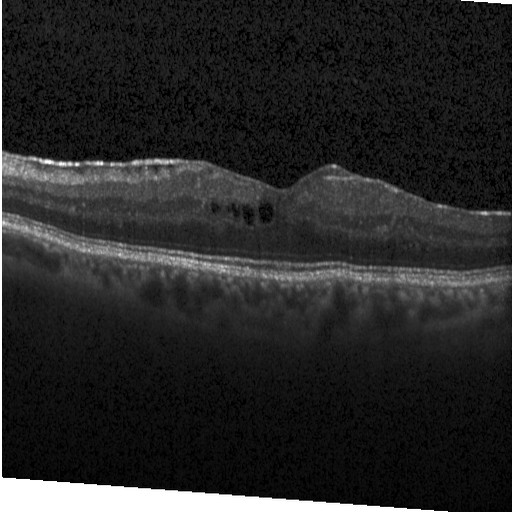
OCT B-scan. The scan shows diabetic macular edema.